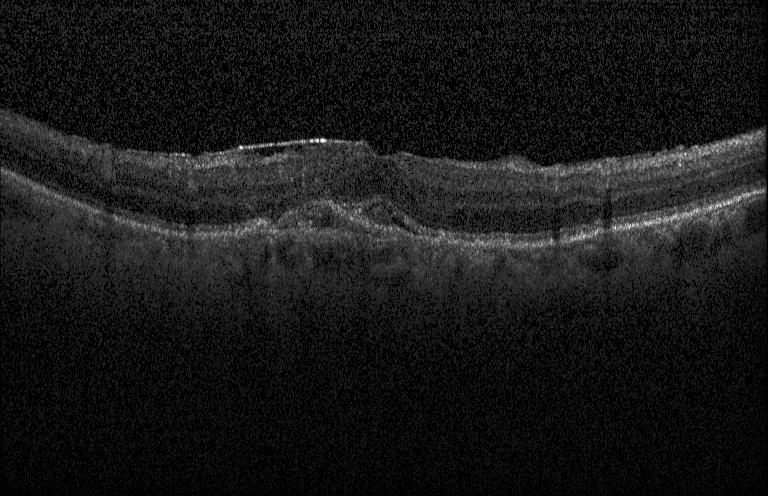 Optical coherence tomography B-scan, macular scan — Impression: a choroidal neovascular membrane.